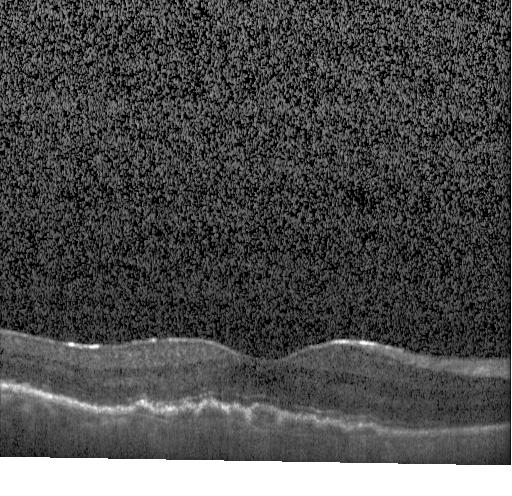 Heidelberg Spectralis OCT system; optical coherence tomography B-scan.
The scan shows a choroidal neovascular membrane.